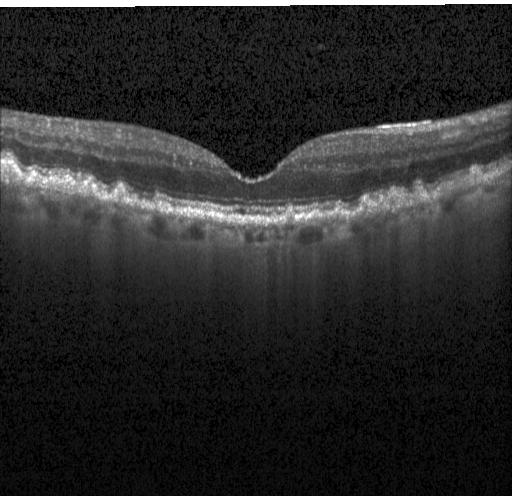
OCT B-scan showing multiple drusen.